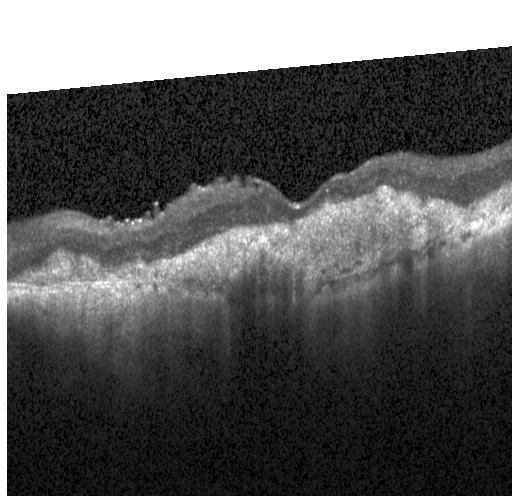
Instrument: Heidelberg Spectralis. Through the macula. Optical coherence tomography B-scan. SD-OCT. Assessment: a choroidal neovascular membrane.